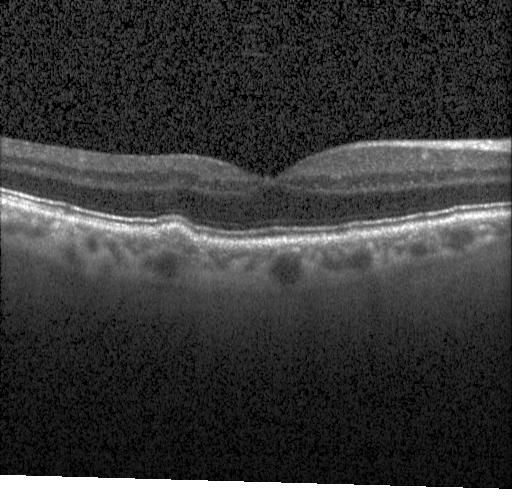 Retinal OCT cross-section — Macular OCT: sub-RPE drusenoid deposits.